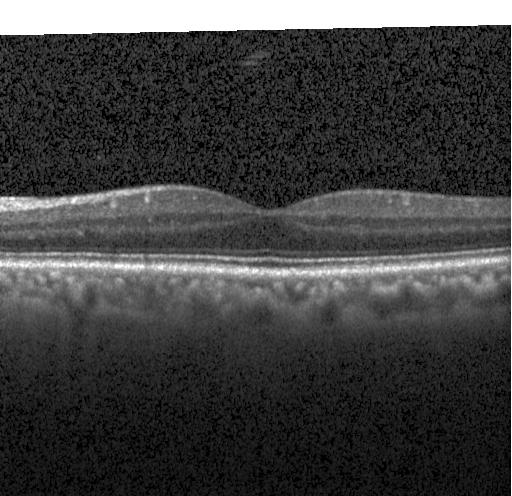

Optical coherence tomography B-scan · macular scan · SD-OCT — Assessment: no choroidal neovascularization, diabetic macular edema, or drusen.